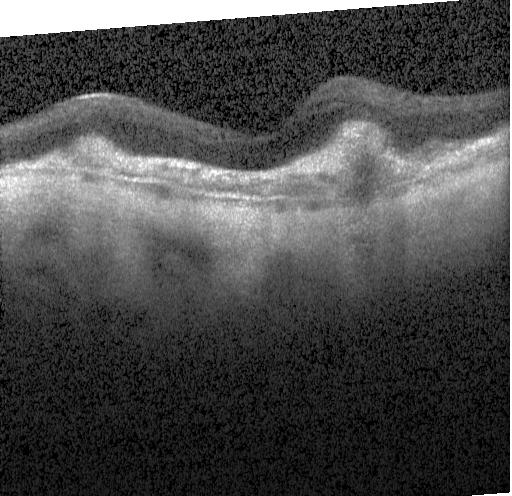
Optical coherence tomography B-scan; spectral-domain OCT; instrument: Heidelberg Spectralis — Assessment: a choroidal neovascular membrane.